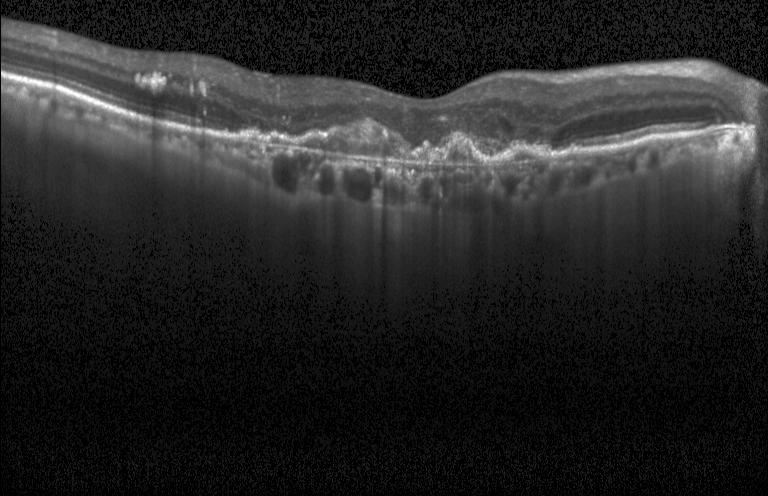 Optical coherence tomography B-scan — Diagnosis: a choroidal neovascular membrane.